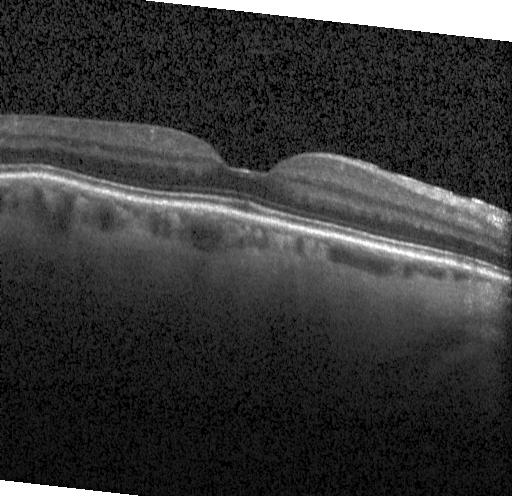

Heidelberg Spectralis. Through the macula. OCT B-scan. Spectral-domain optical coherence tomography.
The scan shows neither CNV, DME, nor drusen.